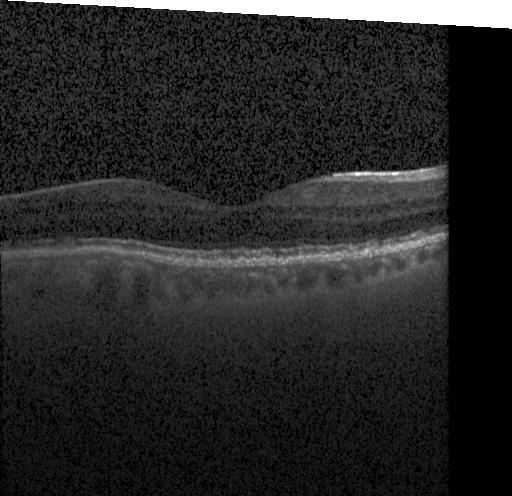
Macular OCT demonstrating no choroidal neovascularization, no diabetic macular edema, and no drusen.